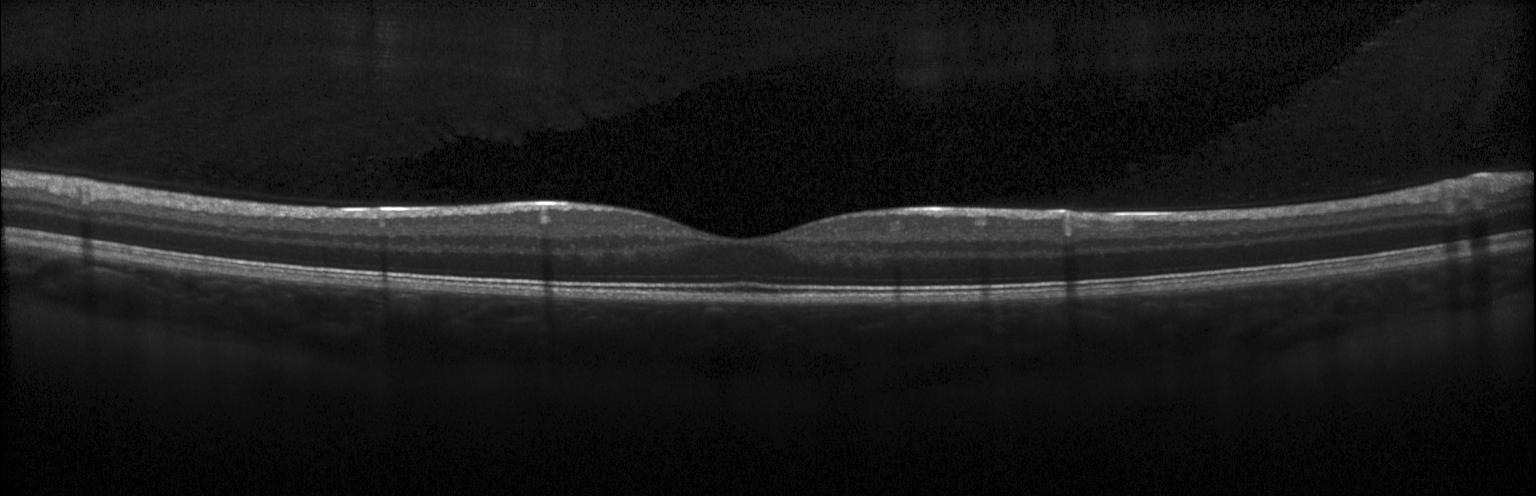
OCT line scan — Diagnosis: no choroidal neovascularization, no diabetic macular edema, and no drusen.